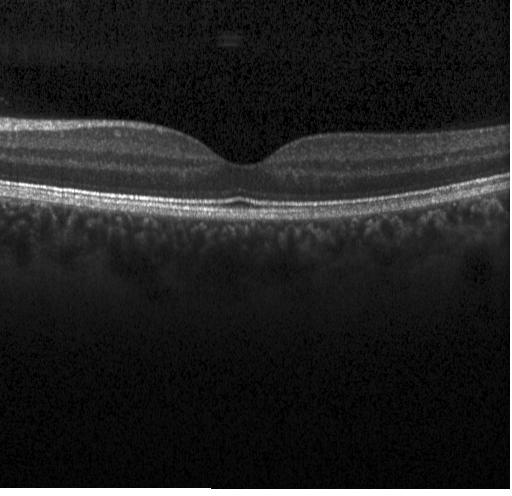
OCT finding: no choroidal neovascularization, diabetic macular edema, or drusen.